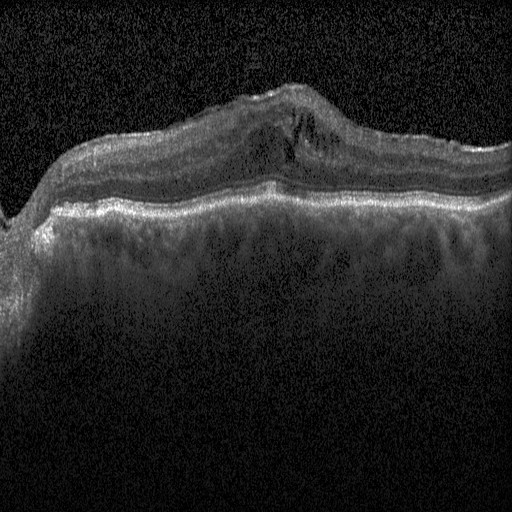
This B-scan demonstrates diabetic macular edema (DME).